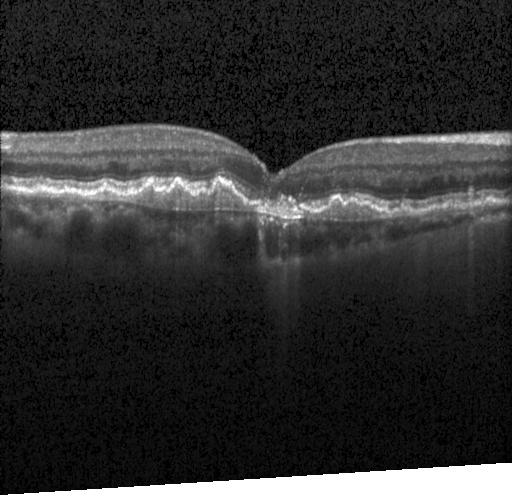
Instrument: Heidelberg Spectralis. Through the macula. Retinal OCT cross-section — Impression: CNV.